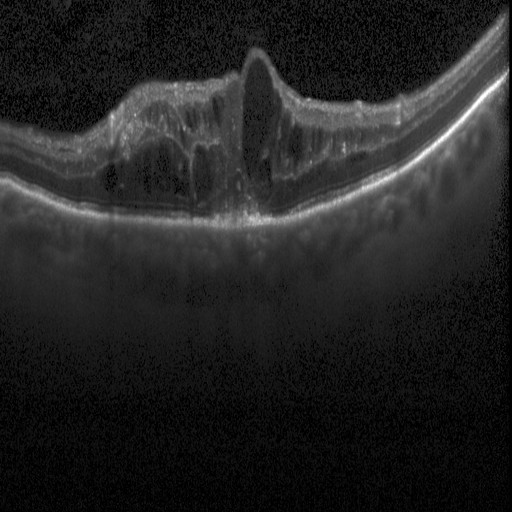
Diabetic macular edema (DME).